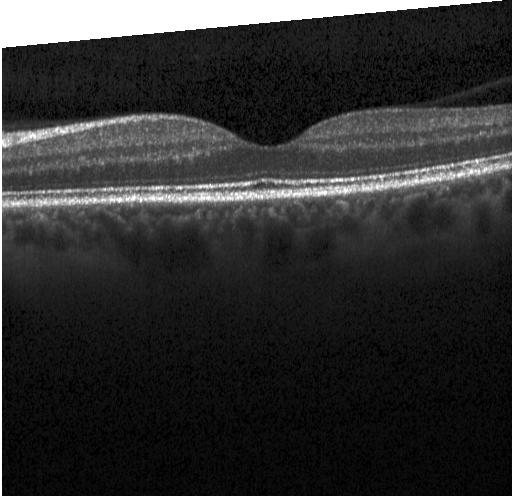

Impression: no evidence of choroidal neovascularization, diabetic macular edema, or drusen.